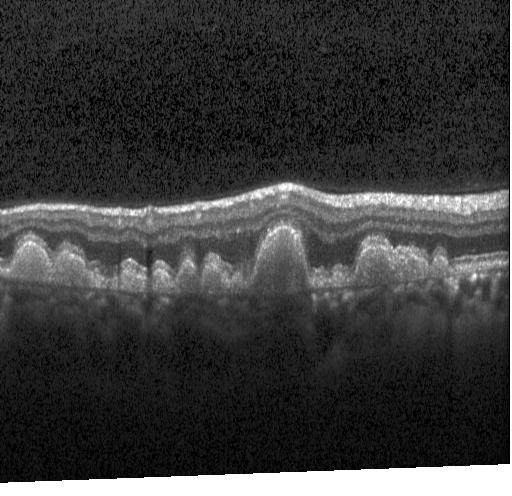

Retinal OCT B-scan — OCT finding: multiple drusen.